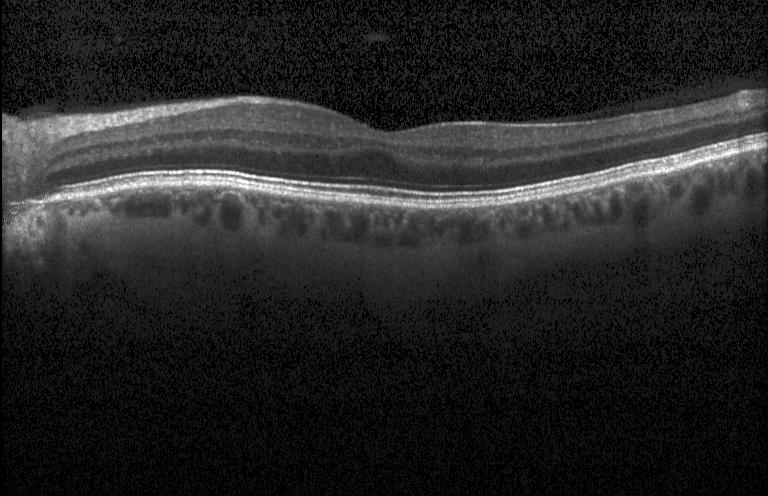

OCT scan showing neither CNV, DME, nor drusen.